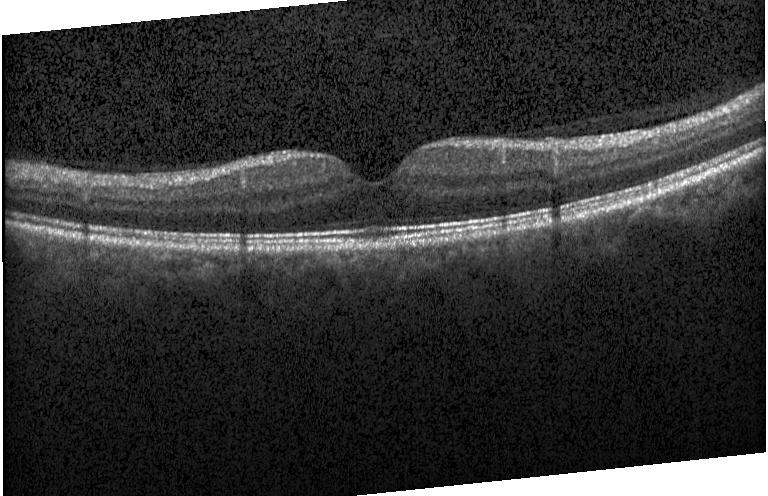
Horizontal scan through the fovea. Heidelberg Spectralis OCT system. Spectral-domain optical coherence tomography. OCT line scan.
Dx: no choroidal neovascularization, no diabetic macular edema, and no drusen.